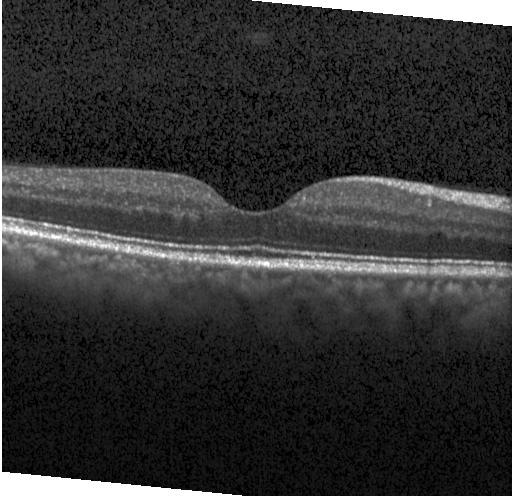

Centered on the fovea. SD-OCT. OCT line scan. Heidelberg Spectralis. This B-scan demonstrates no choroidal neovascularization, no diabetic macular edema, and no drusen.